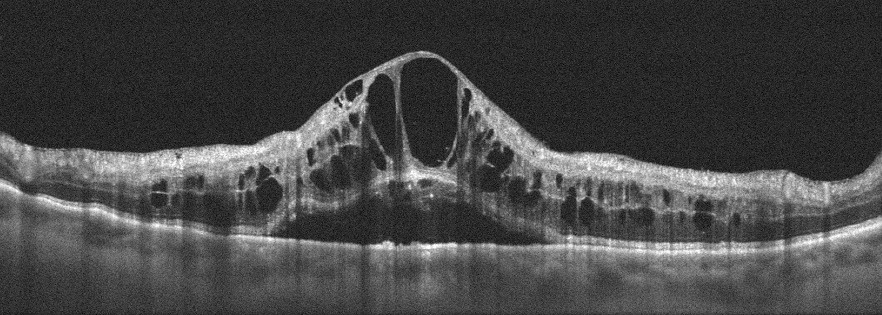 OCT B-scan, macular scan. Diagnosis: retinal vein occlusion (RVO).